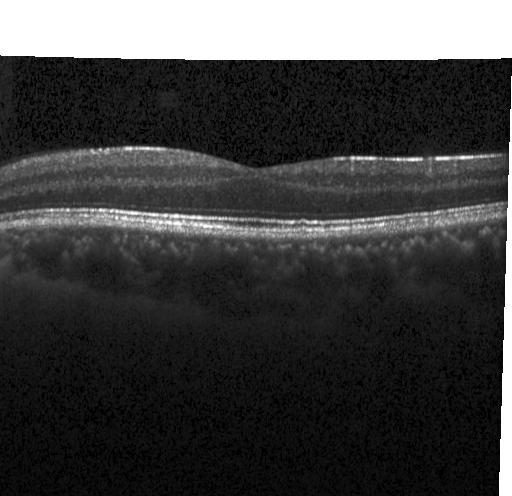
Macular OCT: neither choroidal neovascularization, diabetic macular edema, nor drusen.